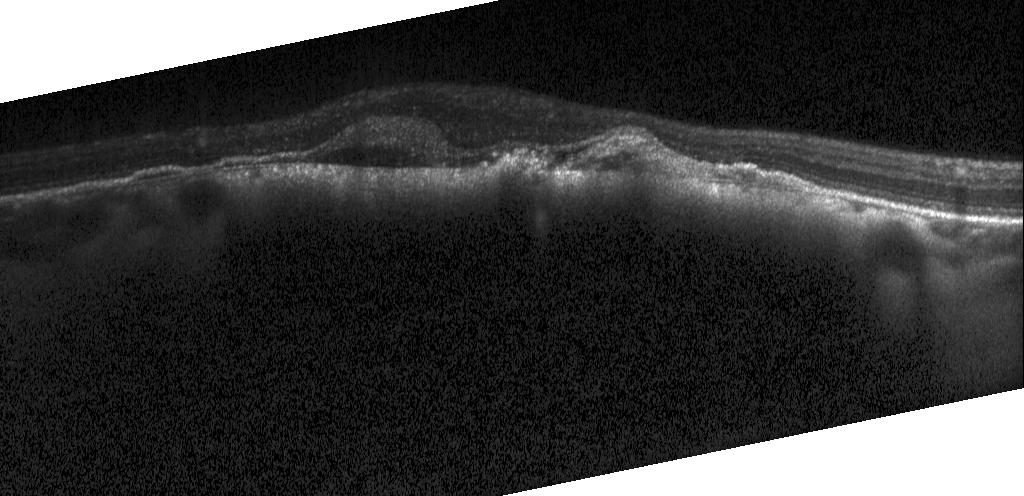

Macular OCT: choroidal neovascularization.